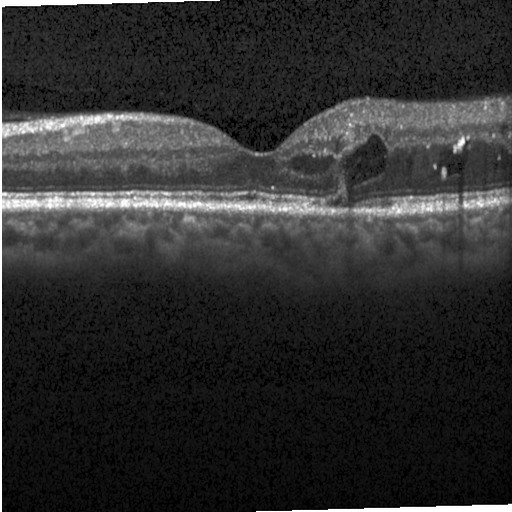

Dx: diabetic macular edema (DME).